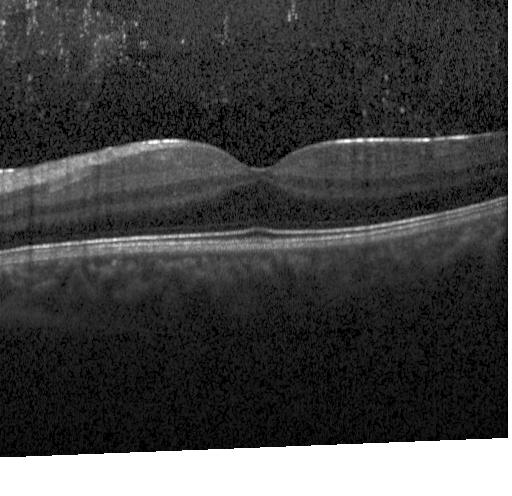 Horizontal scan through the fovea; Heidelberg Spectralis; optical coherence tomography scan — The scan shows no evidence of choroidal neovascularization, diabetic macular edema, or drusen.